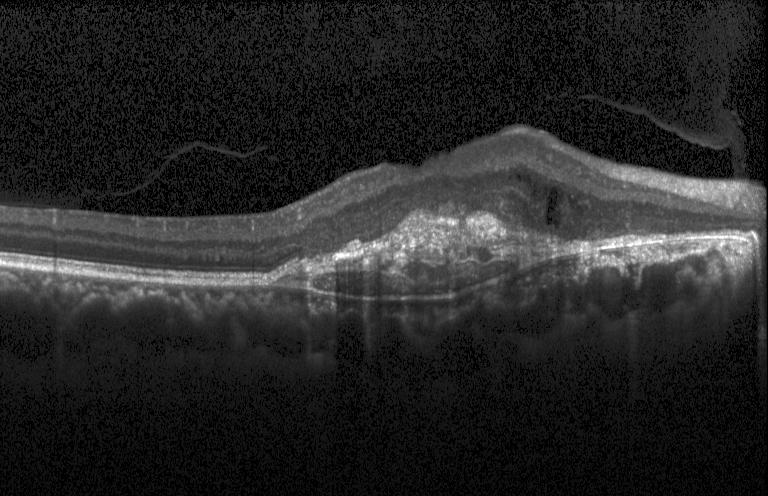

Macular OCT demonstrating a choroidal neovascular membrane.